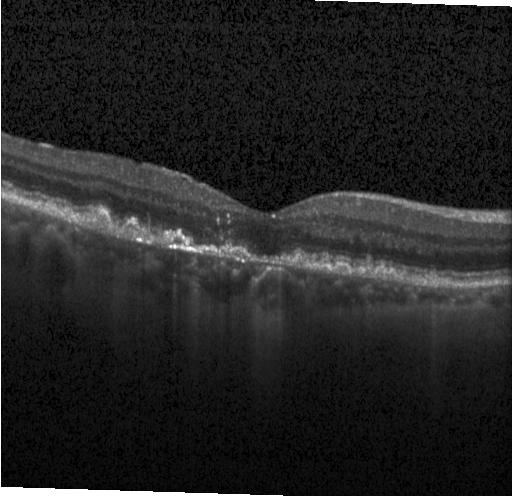

SD-OCT. Retinal OCT cross-section. Heidelberg Spectralis OCT system.
The scan shows choroidal neovascularization (CNV).